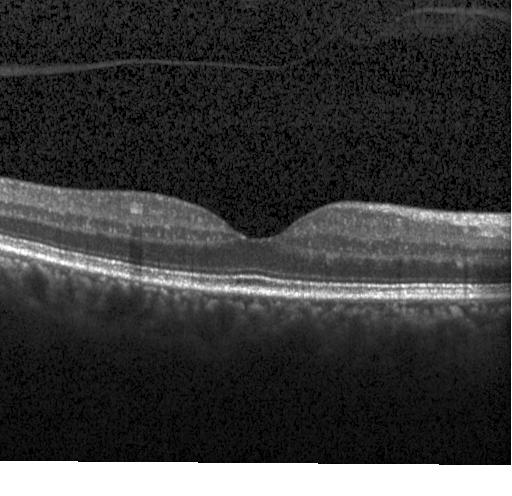

Spectral-domain OCT; instrument: Heidelberg Spectralis; OCT B-scan — Dx: no choroidal neovascularization, diabetic macular edema, or drusen.